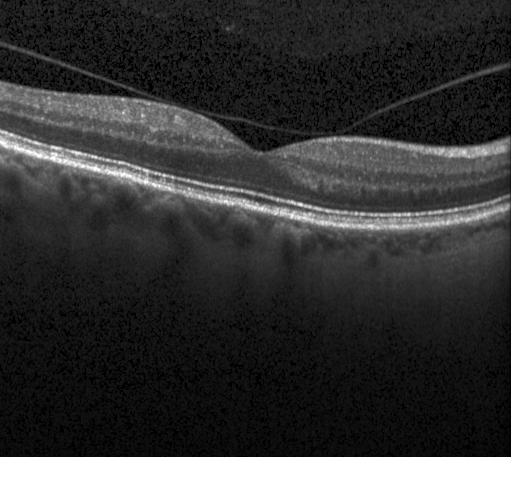
Optical coherence tomography B-scan. Macular scan. Heidelberg Spectralis OCT system
Finding: no choroidal neovascularization, diabetic macular edema, or drusen.